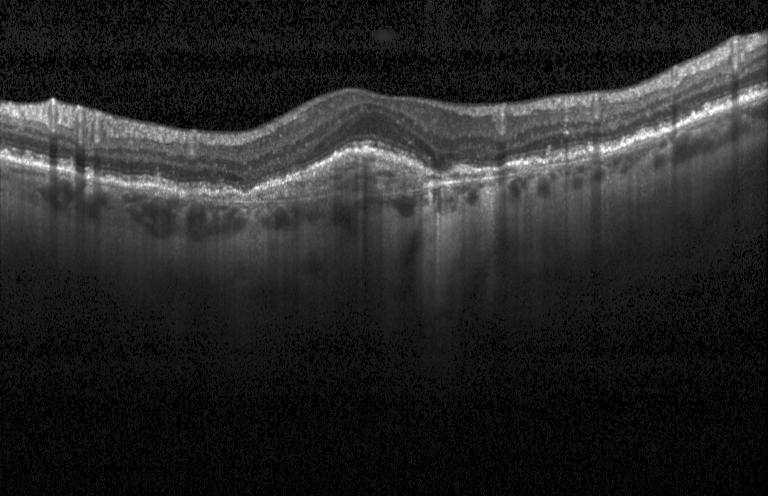 Optical coherence tomography B-scan, spectral-domain optical coherence tomography, centered on the fovea, Heidelberg Spectralis OCT system. Diagnosis: a choroidal neovascular membrane.